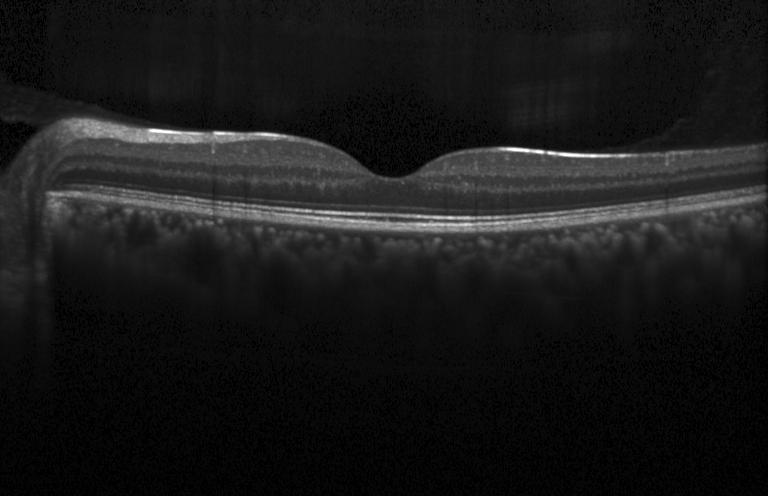 Diagnosis: no choroidal neovascularization, diabetic macular edema, or drusen.